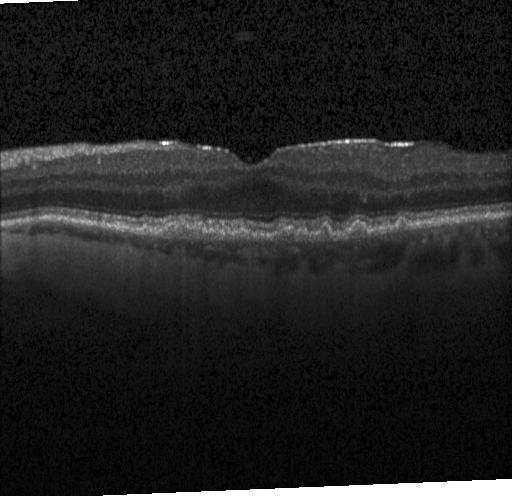 SD-OCT · Heidelberg Spectralis OCT system · retinal OCT cross-section · horizontal scan through the fovea.
Finding: drusen.